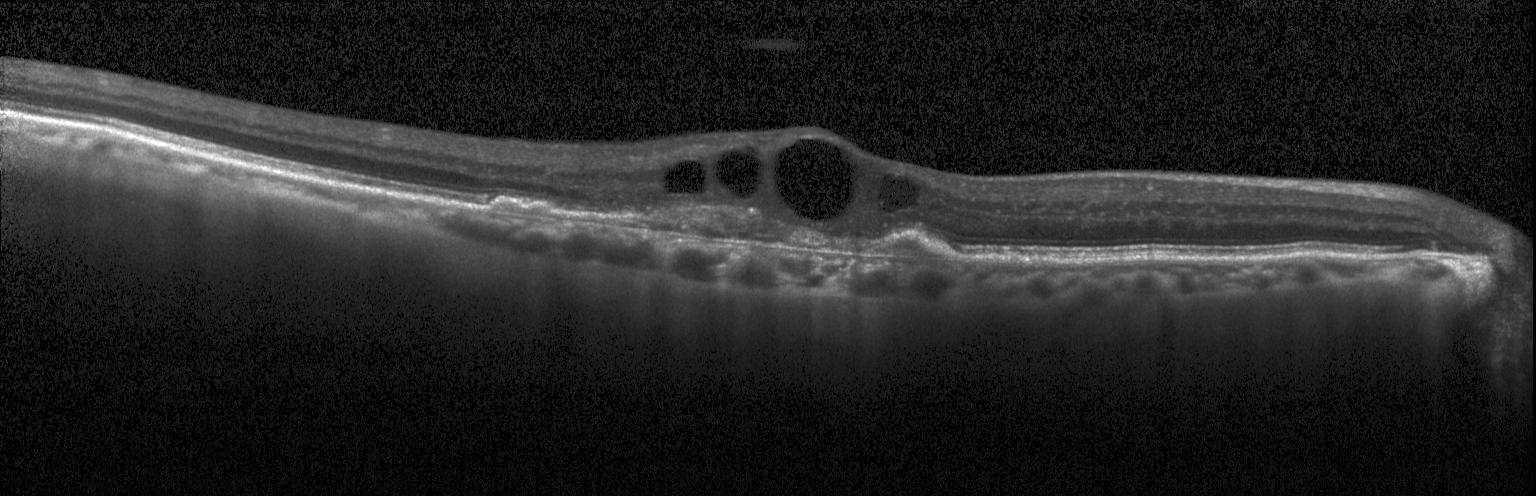
Macular OCT: a choroidal neovascular membrane.